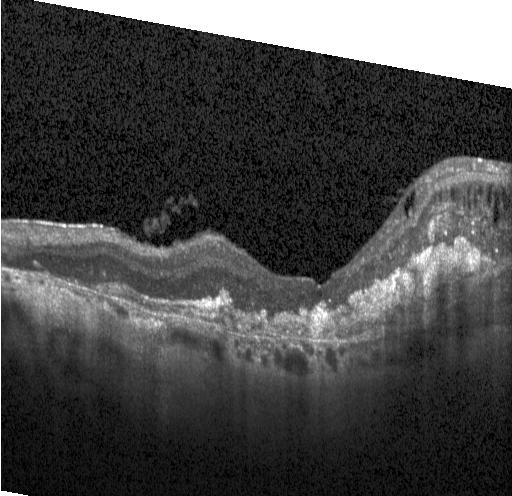
OCT B-scan showing choroidal neovascularization (CNV).